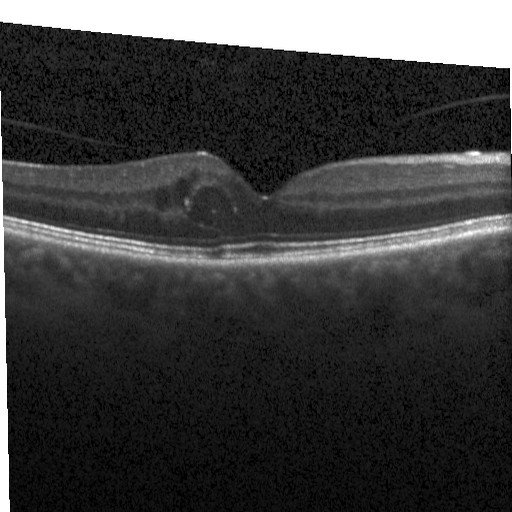
Retinal OCT B-scan. Dx: diabetic macular edema.